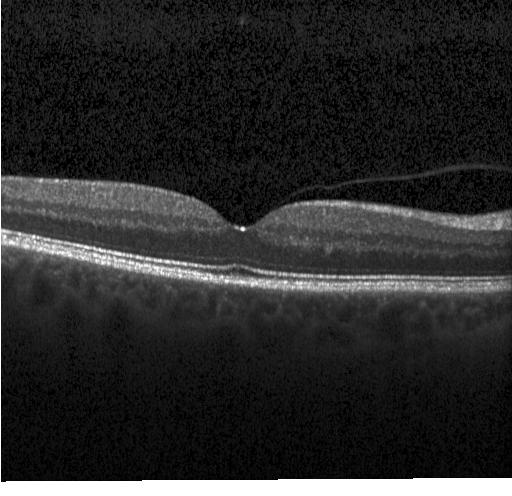

Assessment: no evidence of choroidal neovascularization, diabetic macular edema, or drusen.